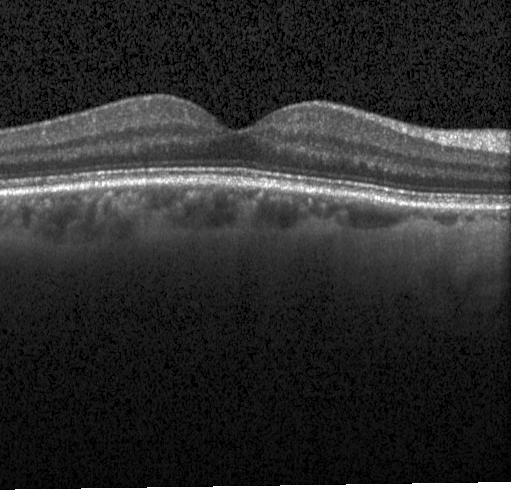

OCT B-scan. Horizontal scan through the fovea.
No evidence of choroidal neovascularization, diabetic macular edema, or drusen.